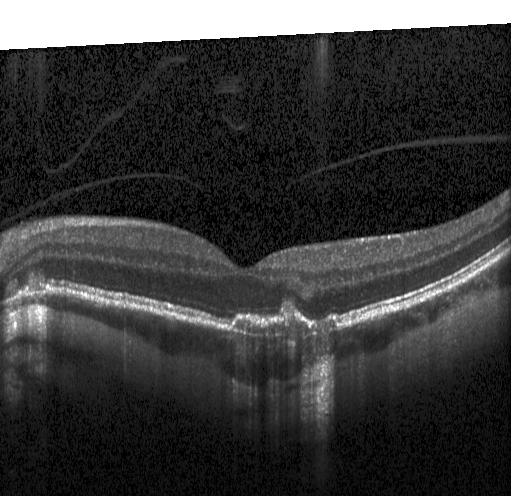

OCT B-scan showing choroidal neovascularization.